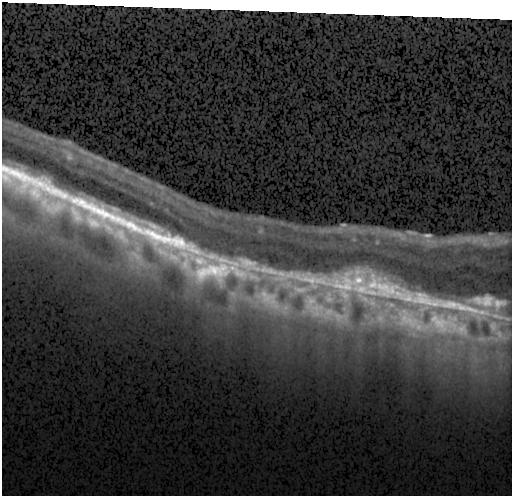
Assessment: CNV.